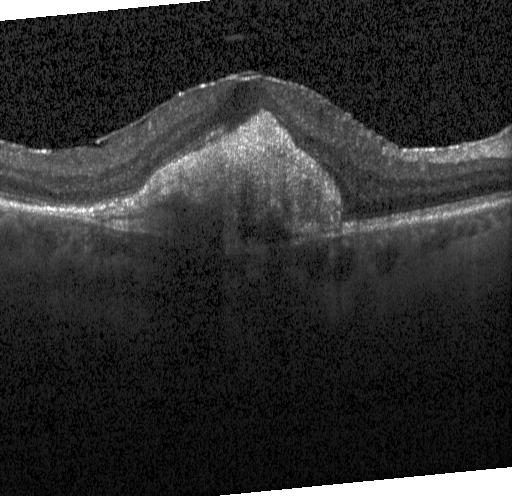

Dx: CNV.